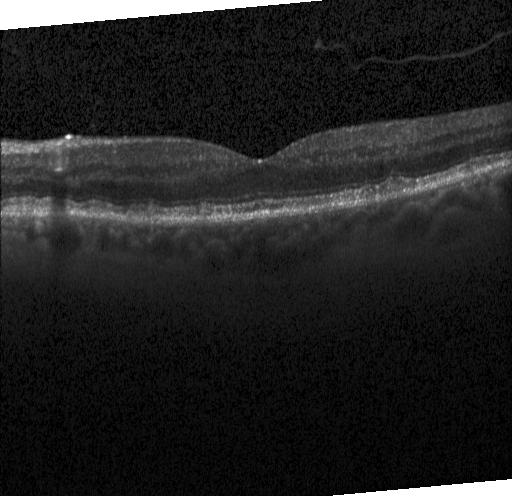
OCT B-scan.
Assessment: multiple drusen.